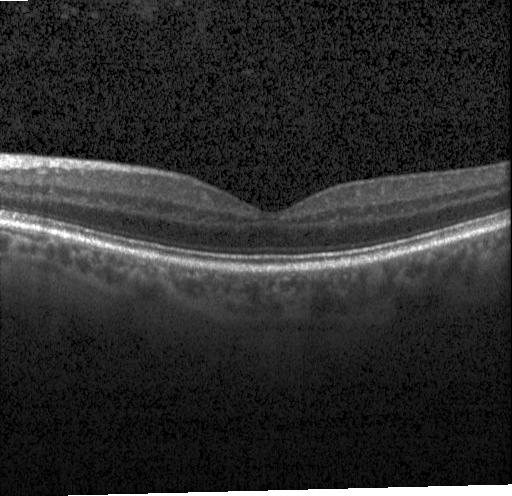

Retinal OCT cross-section; instrument: Heidelberg Spectralis; spectral-domain OCT.
Macular OCT: no choroidal neovascularization, no diabetic macular edema, and no drusen.